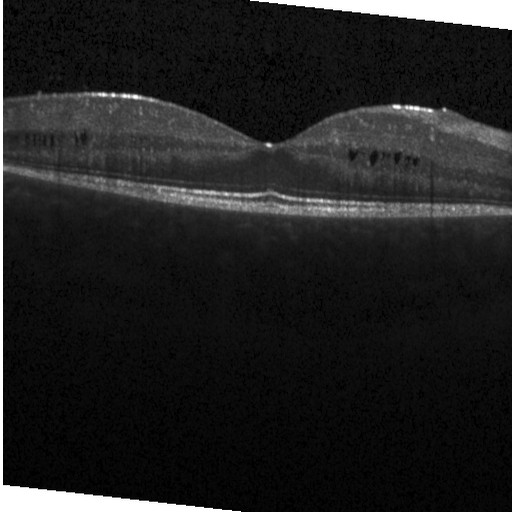
Spectral-domain optical coherence tomography, OCT line scan — Diagnosis: diabetic macular edema.